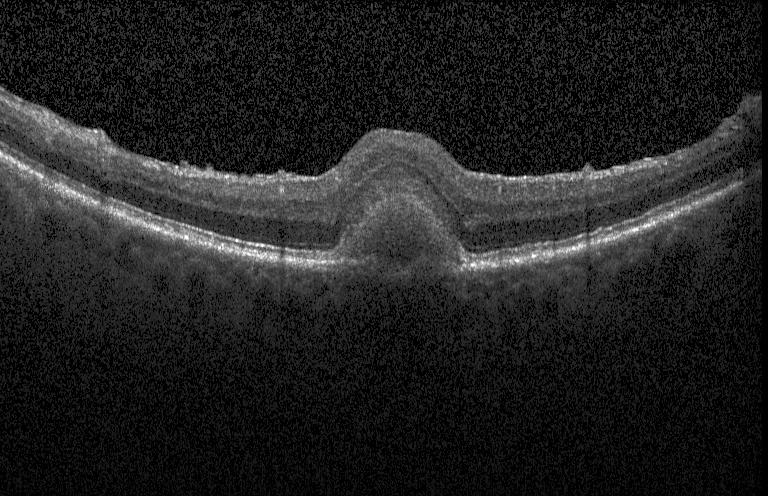 Spectral-domain optical coherence tomography · Heidelberg Spectralis · retinal OCT cross-section. A choroidal neovascular membrane.